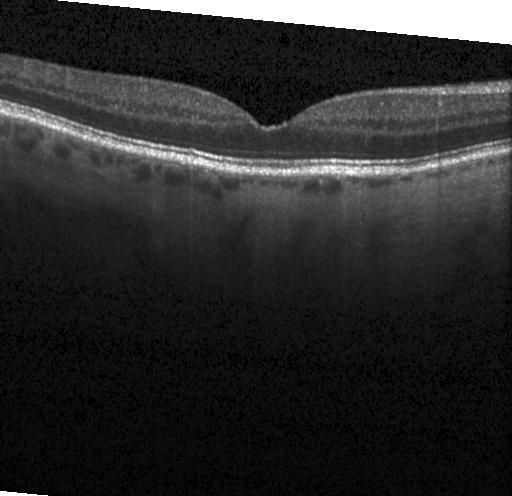 Optical coherence tomography B-scan. Dx: neither choroidal neovascularization, diabetic macular edema, nor drusen.